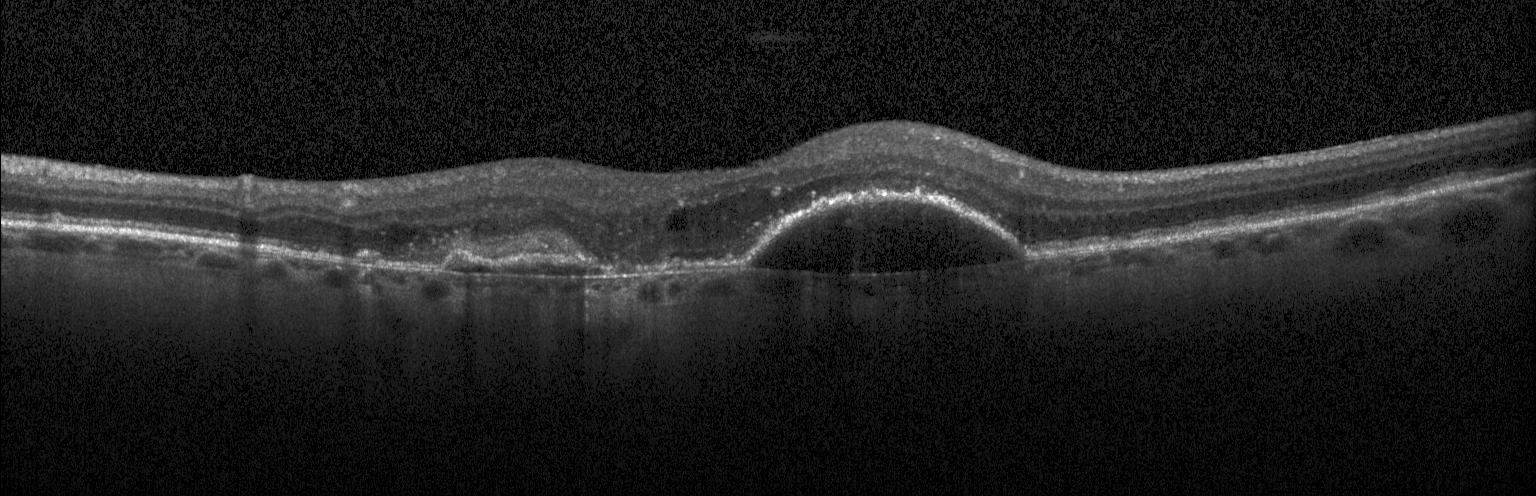

OCT B-scan — Dx: a choroidal neovascular membrane.